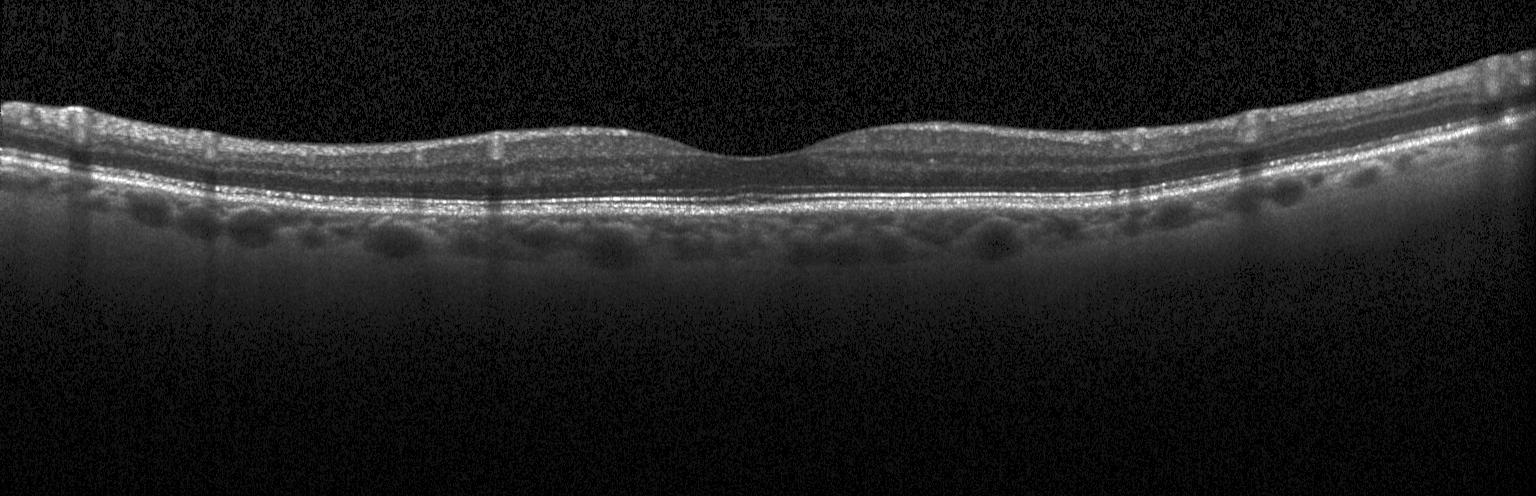 Spectral-domain OCT. Optical coherence tomography scan. Macular scan. Assessment: no choroidal neovascularization, diabetic macular edema, or drusen.